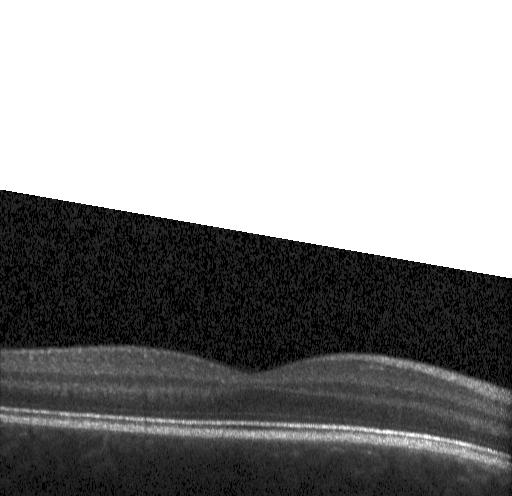

Diagnosis: neither choroidal neovascularization, diabetic macular edema, nor drusen.